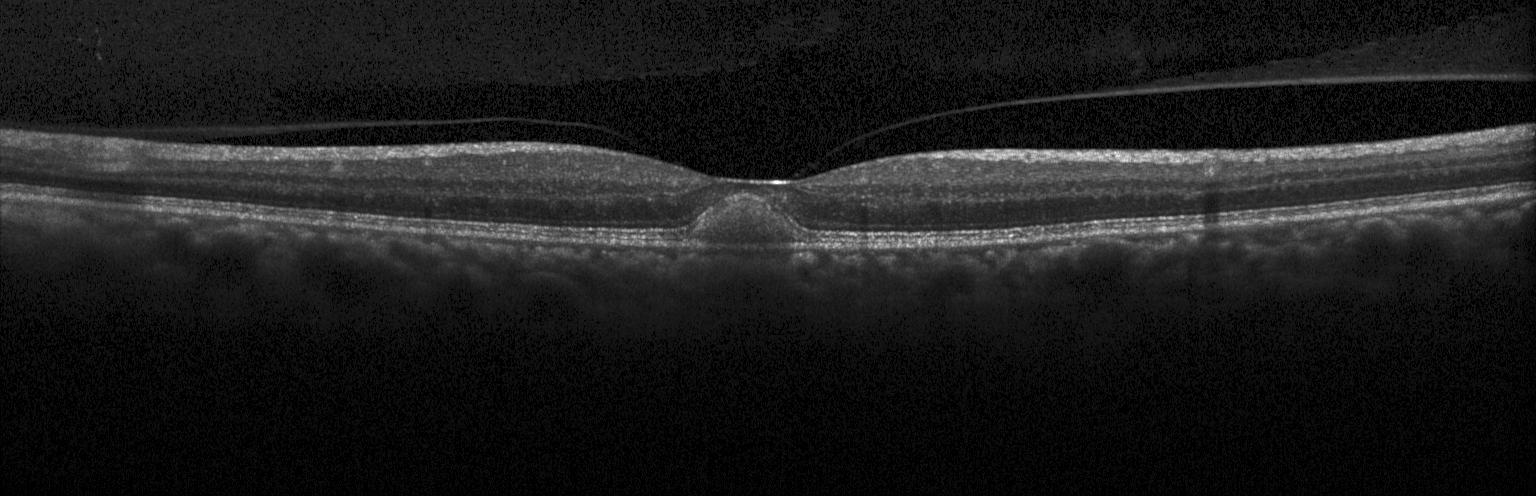 OCT line scan.
A choroidal neovascular membrane.